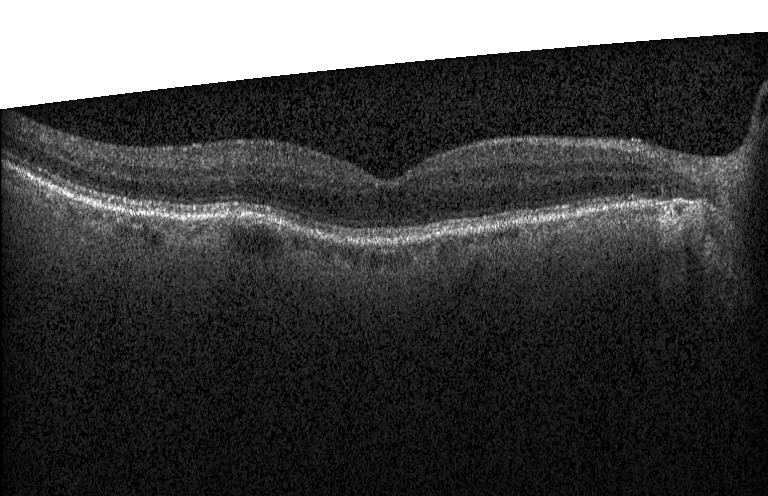

Retinal OCT cross-section.
Assessment: no choroidal neovascularization, diabetic macular edema, or drusen.